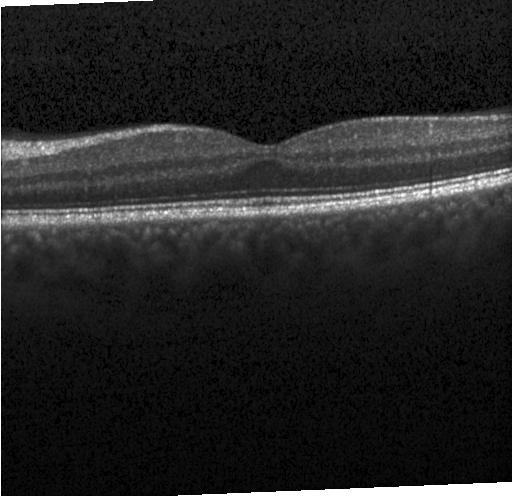 Impression: no evidence of choroidal neovascularization, diabetic macular edema, or drusen.